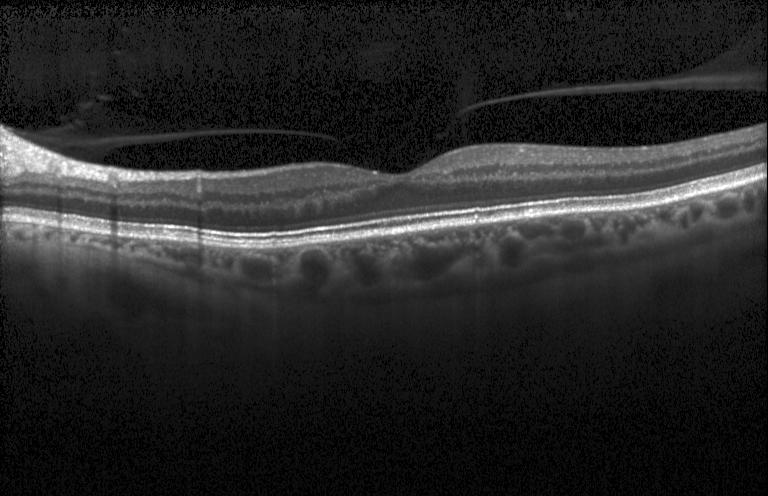 Heidelberg Spectralis · spectral-domain OCT · retinal OCT cross-section.
Diagnosis: no choroidal neovascularization, no diabetic macular edema, and no drusen.